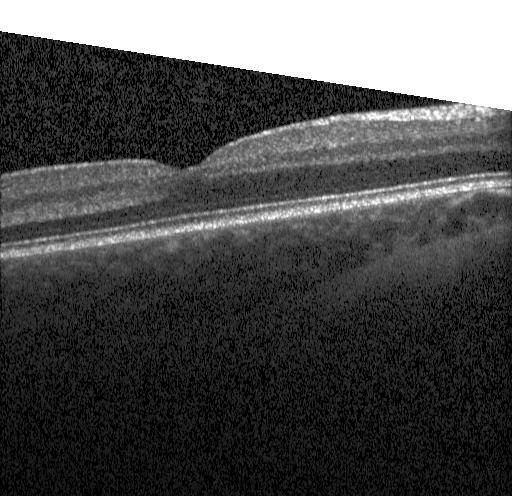

SD-OCT; optical coherence tomography B-scan; through the macula; instrument: Heidelberg Spectralis
Finding: no choroidal neovascularization, diabetic macular edema, or drusen.